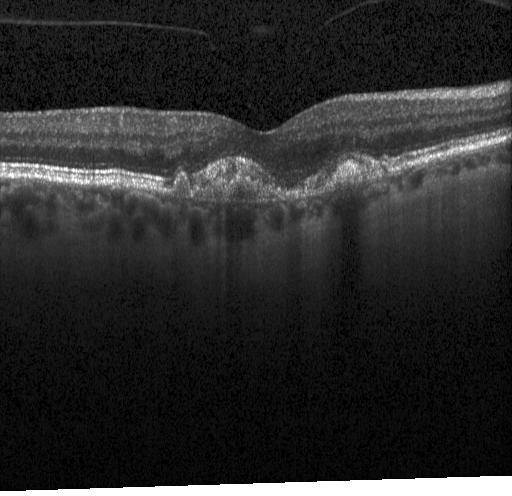 Retinal OCT cross-section — Impression: choroidal neovascularization.